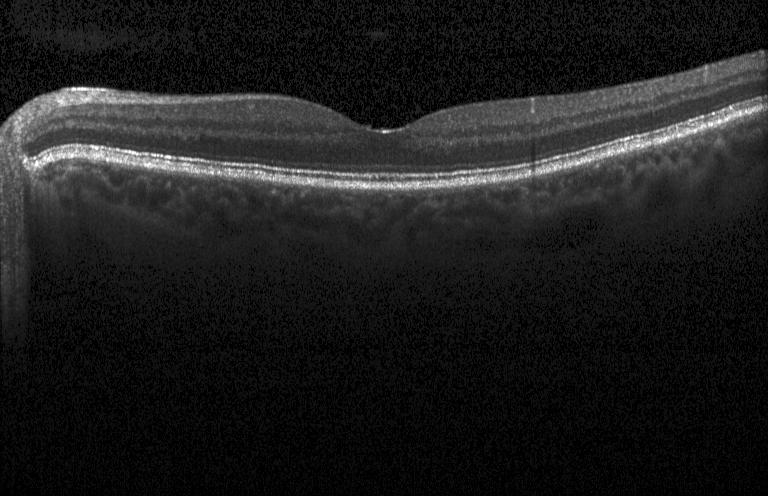 Retinal OCT cross-section showing no evidence of choroidal neovascularization, diabetic macular edema, or drusen.